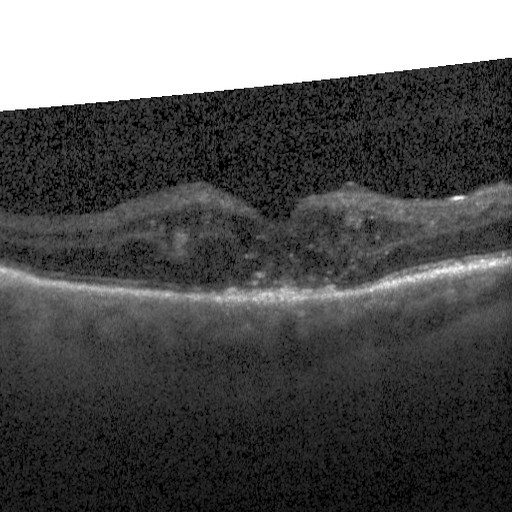

Macular OCT demonstrating diabetic macular edema (DME).